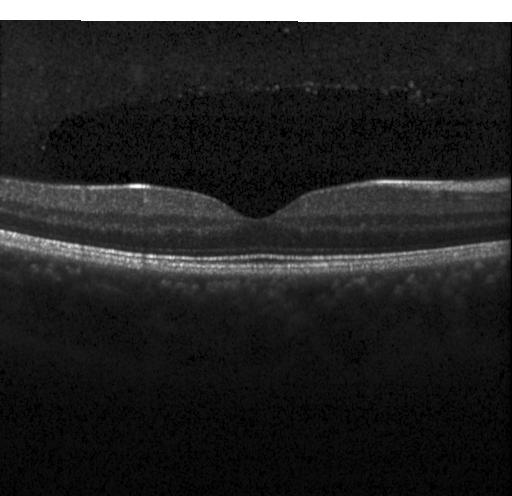
Retinal OCT B-scan · spectral-domain optical coherence tomography · through the macula · acquired on a Heidelberg Spectralis.
Macular OCT: no evidence of choroidal neovascularization, diabetic macular edema, or drusen.